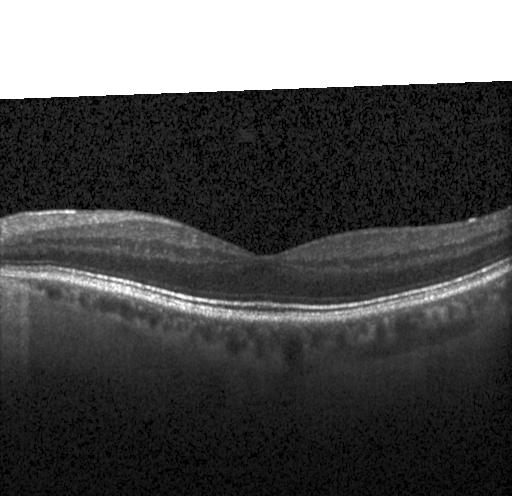
Spectral-domain OCT B-scan: neither choroidal neovascularization, diabetic macular edema, nor drusen.